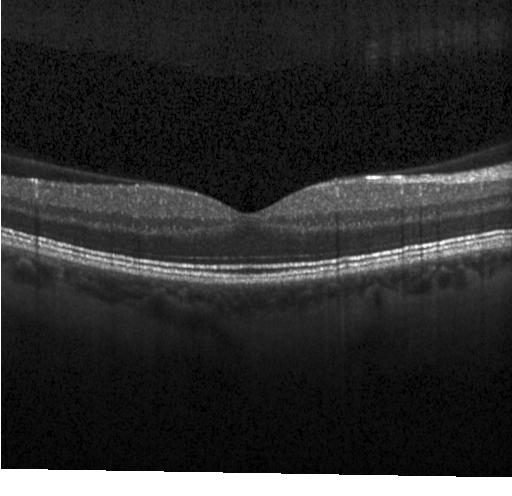
OCT B-scan, horizontal scan through the fovea, Heidelberg Spectralis OCT system, spectral-domain OCT. Dx: no CNV, no DME, and no drusen.